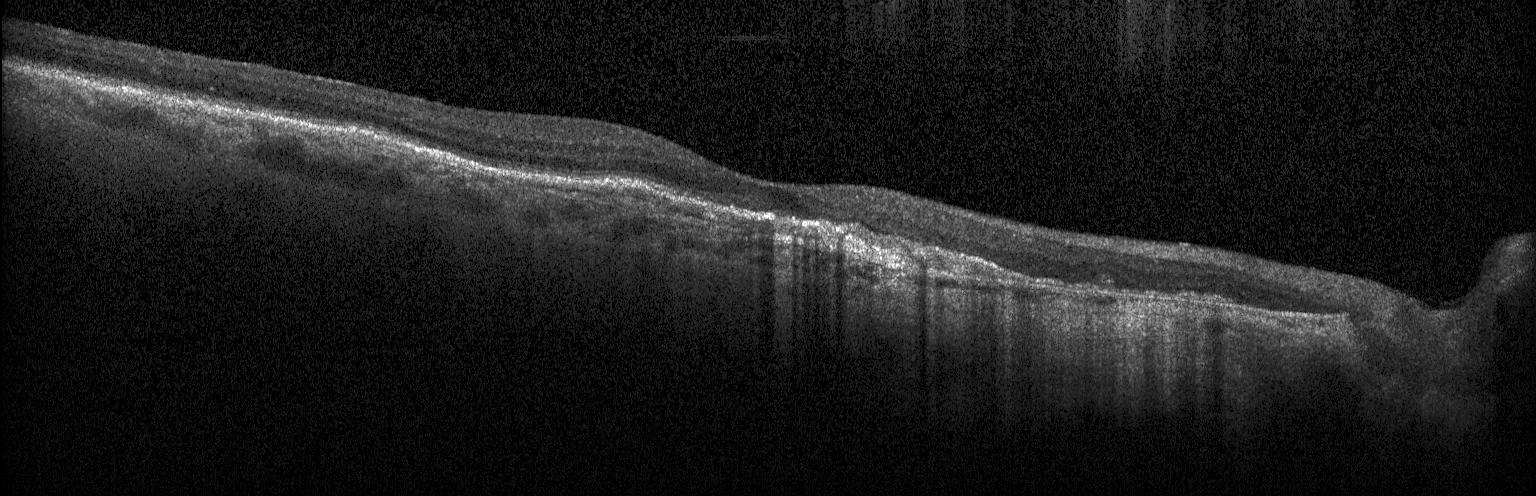
A choroidal neovascular membrane.